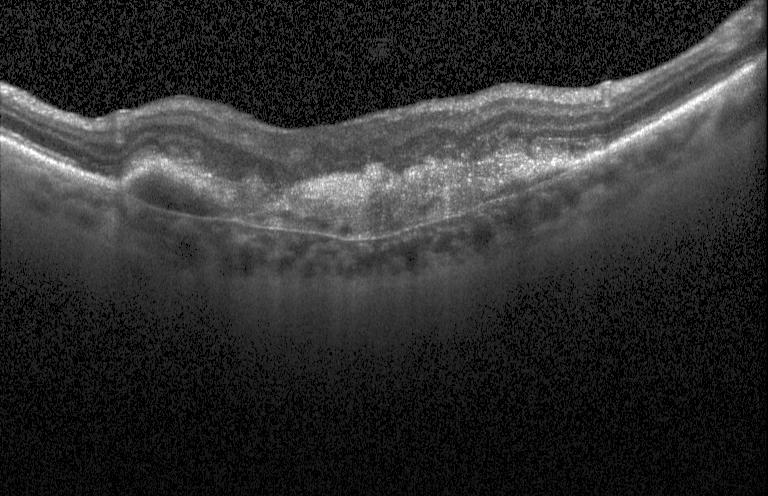

Heidelberg Spectralis OCT system, spectral-domain OCT, retinal OCT B-scan.
Impression: choroidal neovascularization.